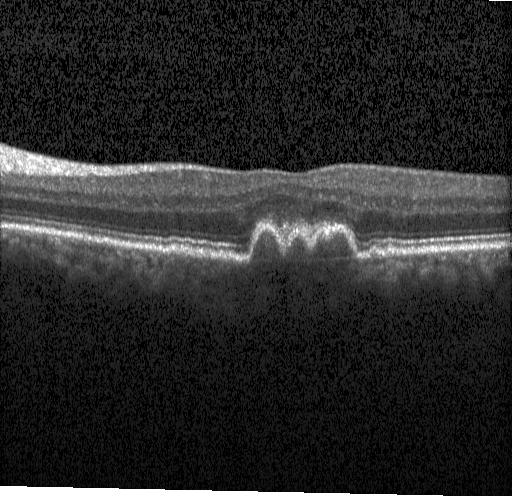

OCT B-scan. Finding: sub-RPE drusenoid deposits.